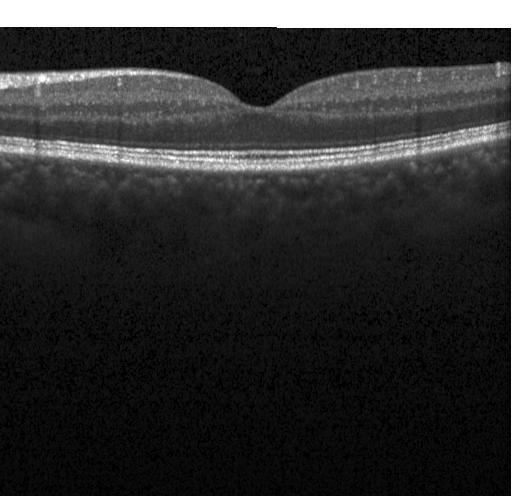 This B-scan demonstrates neither choroidal neovascularization, diabetic macular edema, nor drusen.